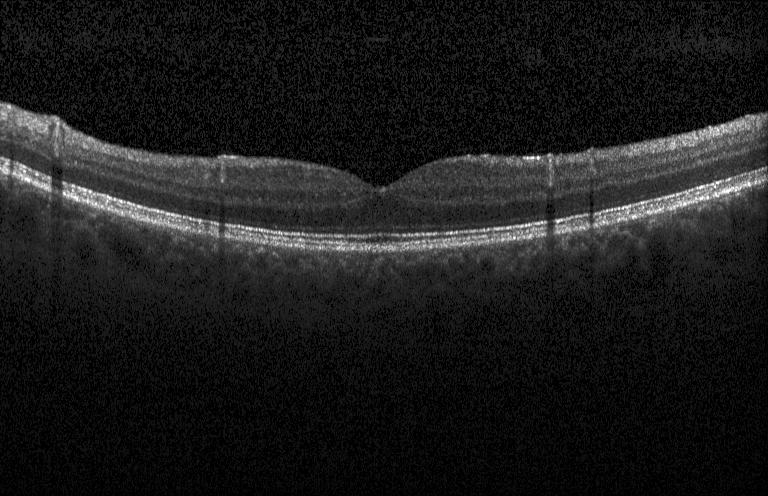

Diagnosis: no choroidal neovascularization, no diabetic macular edema, and no drusen.